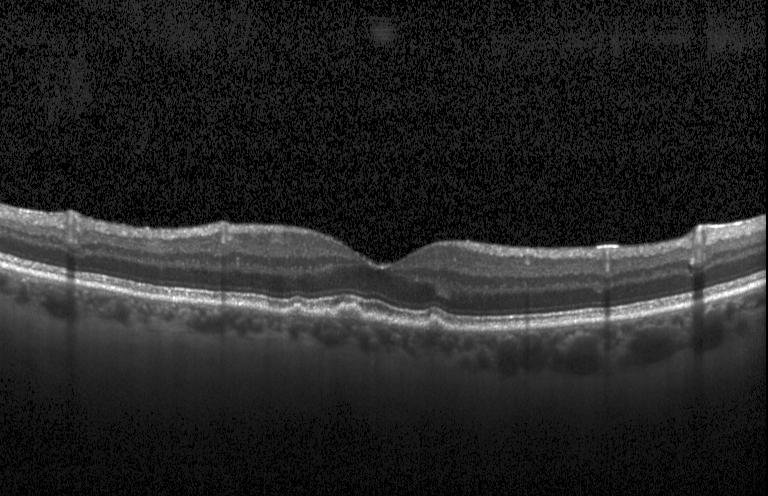
Impression: sub-RPE drusenoid deposits.